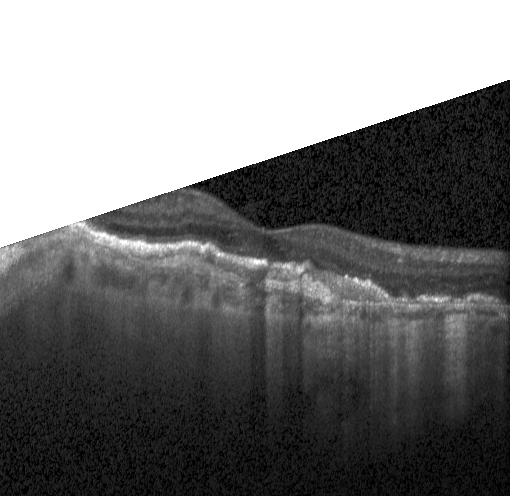

Retinal OCT B-scan · instrument: Heidelberg Spectralis · SD-OCT.
OCT finding: a choroidal neovascular membrane.